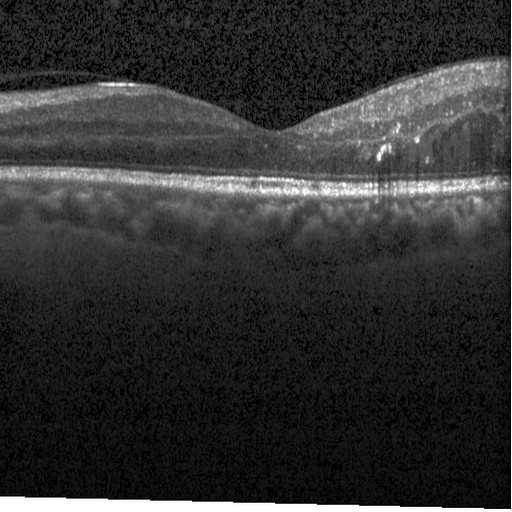 Dx: diabetic macular edema.